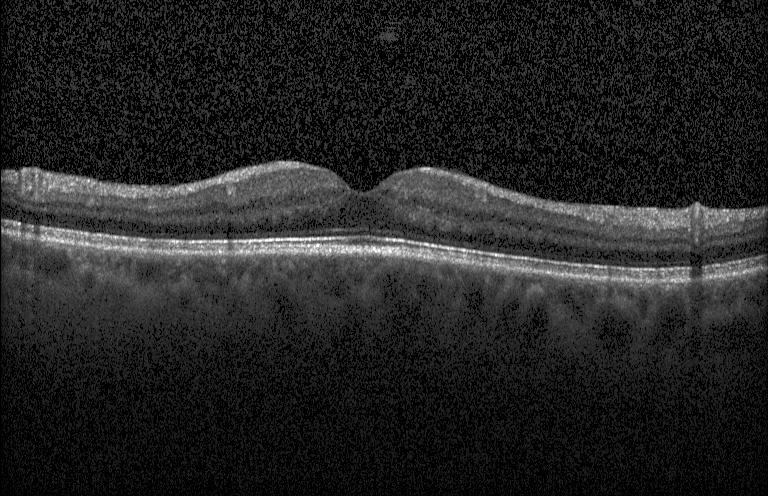
Optical coherence tomography scan, spectral-domain OCT. Assessment: no evidence of choroidal neovascularization, diabetic macular edema, or drusen.